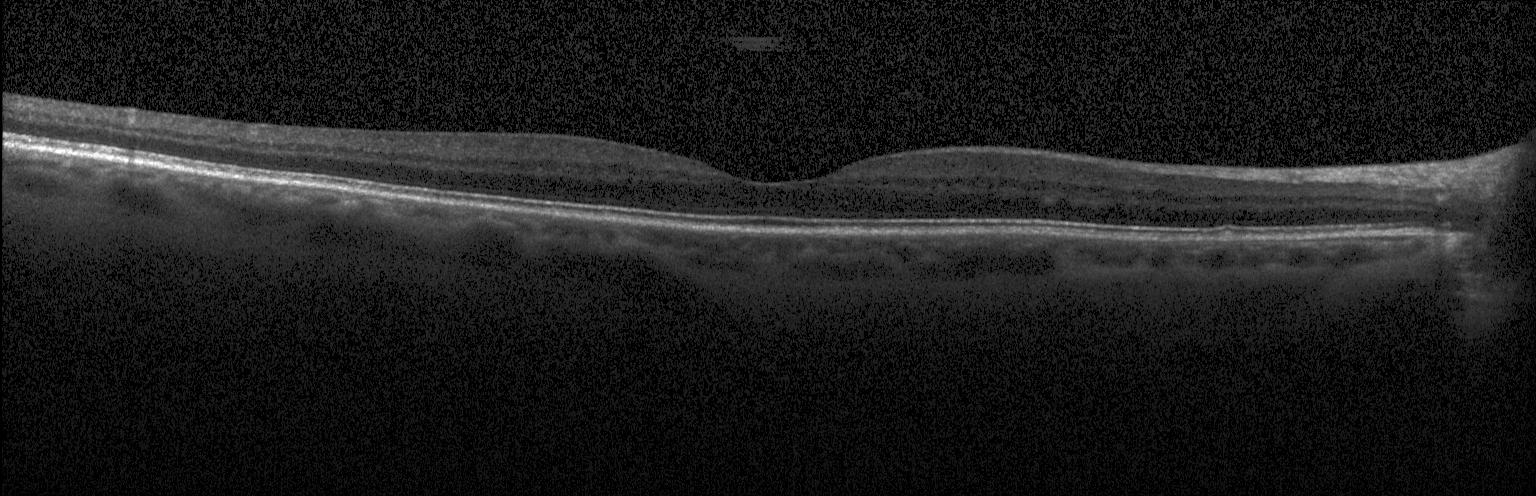

Impression: no evidence of CNV, DME, or drusen.